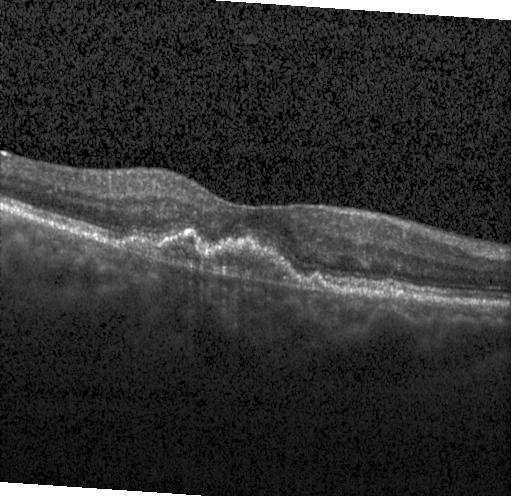 OCT line scan
Choroidal neovascularization.